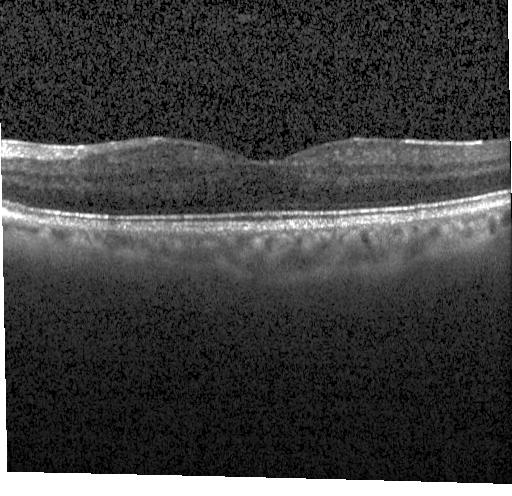
No choroidal neovascularization, no diabetic macular edema, and no drusen.